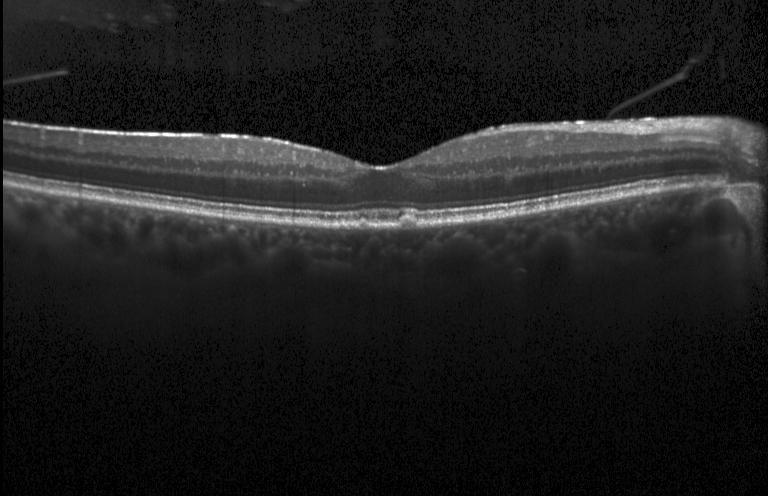
Retinal OCT cross-section showing multiple drusen.